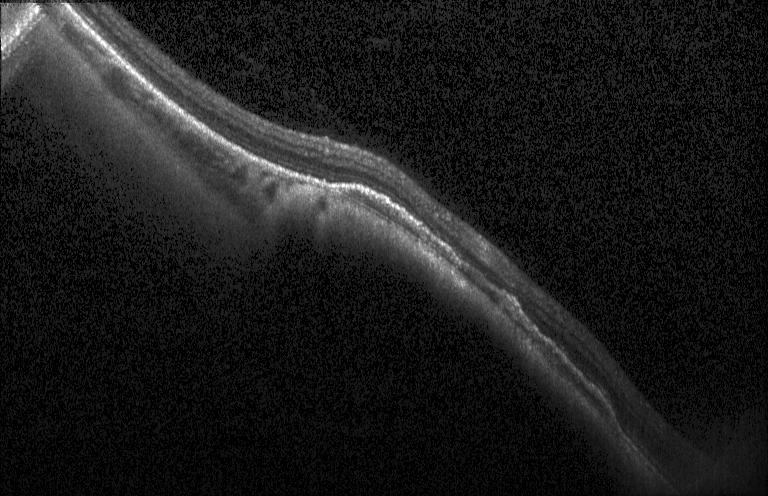

Diagnosis: choroidal neovascularization.